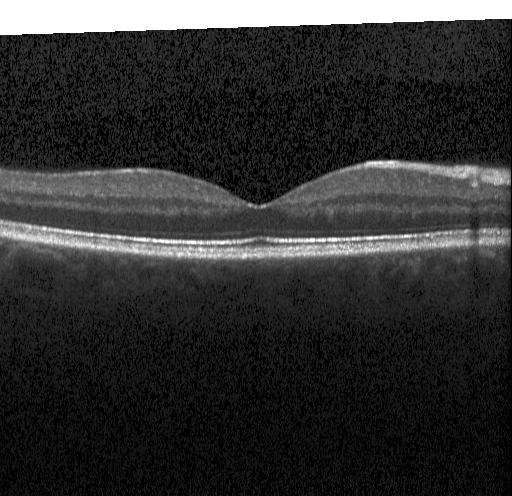

Retinal OCT B-scan · through the macula. The scan shows neither CNV, DME, nor drusen.